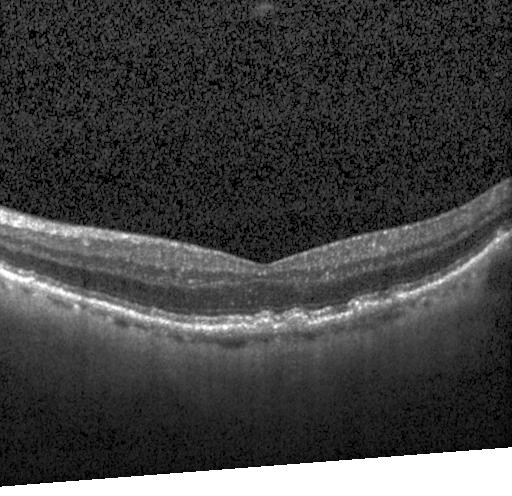

OCT scan showing multiple drusen.